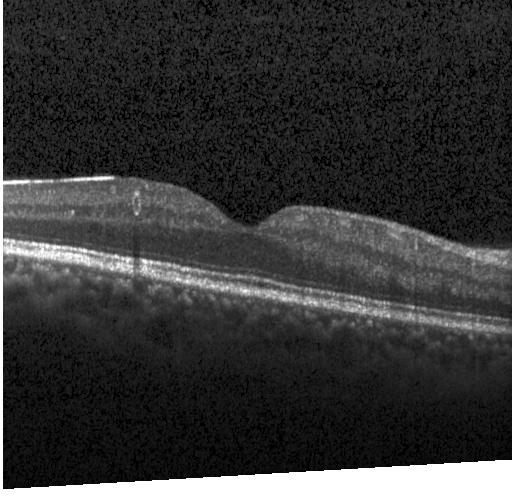

Optical coherence tomography B-scan, SD-OCT. Diagnosis: no CNV, DME, or drusen.